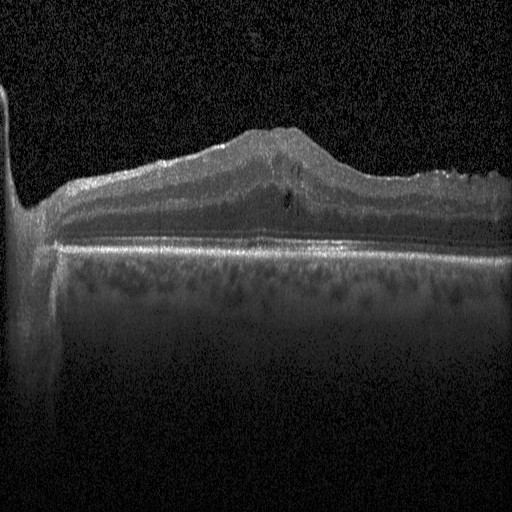

SD-OCT; instrument: Heidelberg Spectralis; retinal OCT cross-section; centered on the fovea.
The scan shows diabetic macular edema (DME).